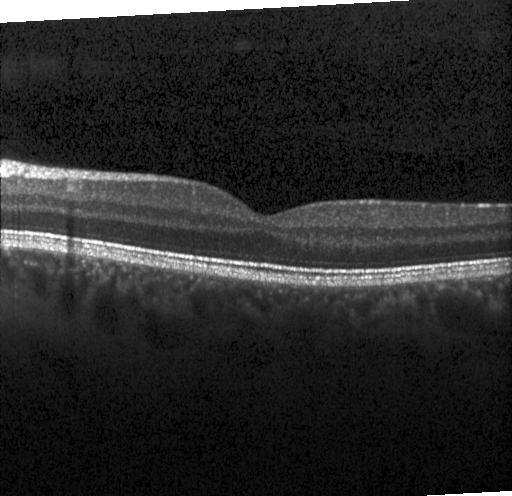

Optical coherence tomography scan.
Dx: neither choroidal neovascularization, diabetic macular edema, nor drusen.